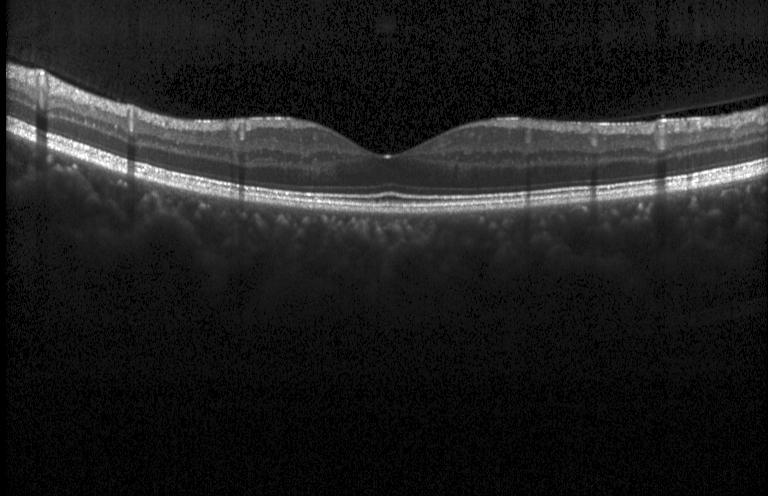

Retinal OCT cross-section — The scan shows no evidence of CNV, DME, or drusen.